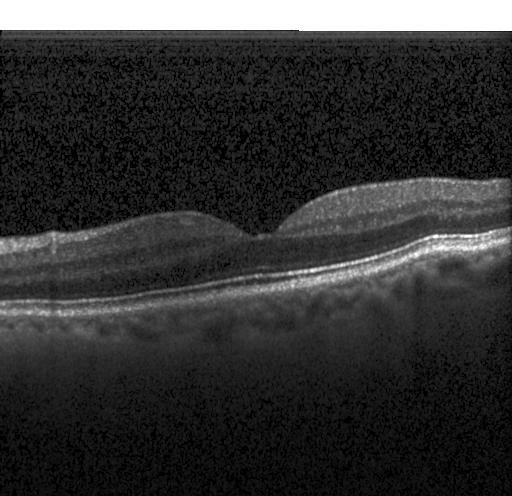

OCT line scan — OCT finding: no evidence of choroidal neovascularization, diabetic macular edema, or drusen.